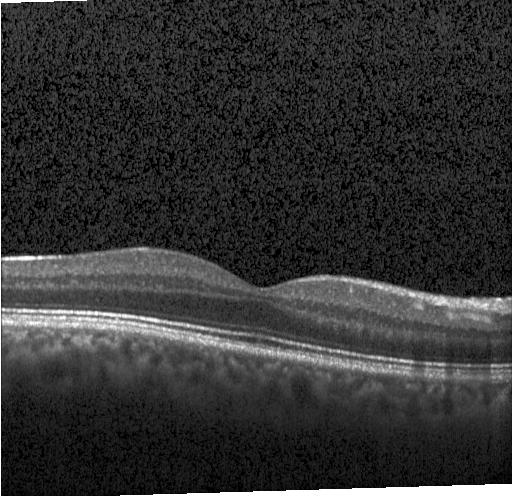

OCT B-scan.
Assessment: no choroidal neovascularization, diabetic macular edema, or drusen.